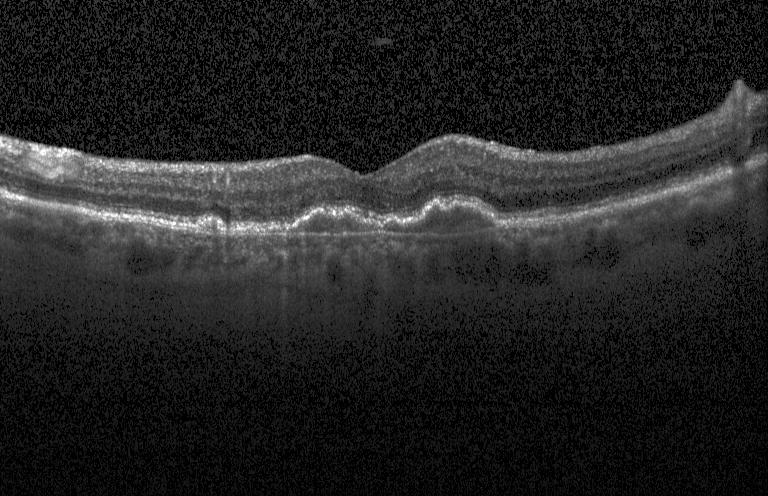 Optical coherence tomography B-scan
A choroidal neovascular membrane.